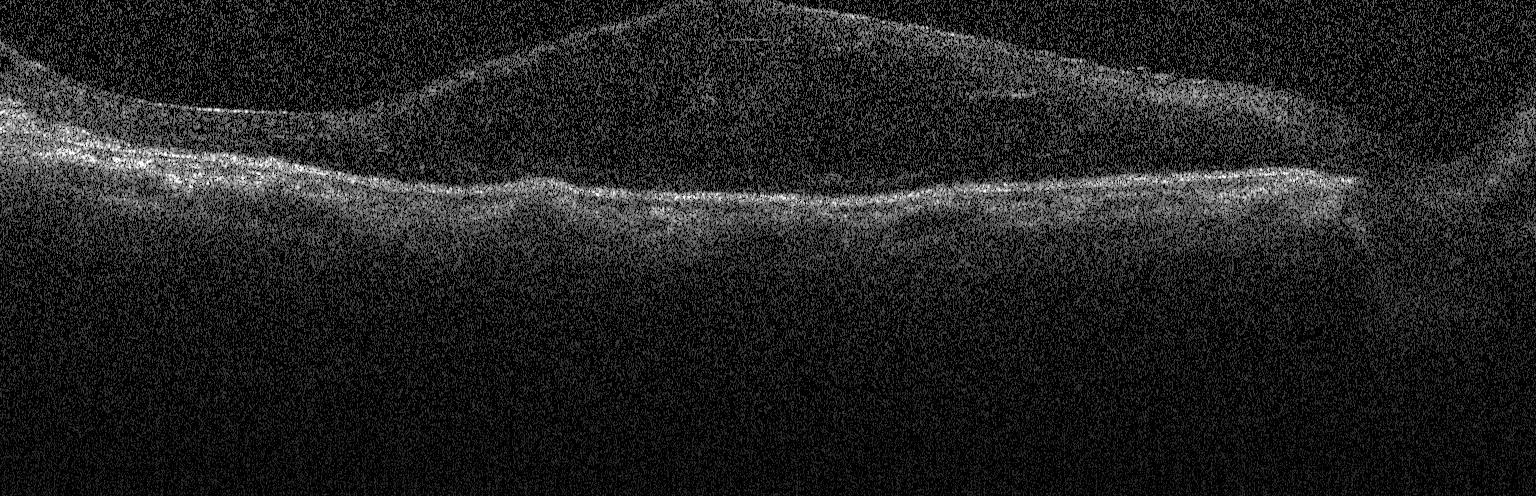
OCT line scan; Heidelberg Spectralis; SD-OCT; centered on the fovea — Assessment: diabetic macular edema.